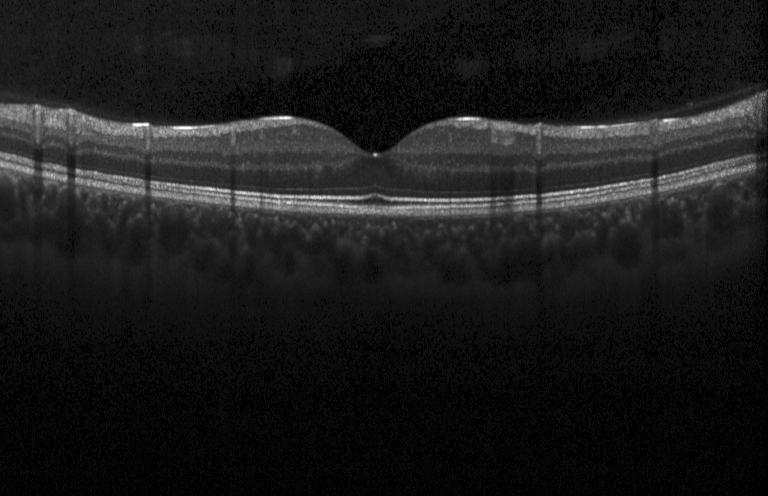

Impression: no evidence of choroidal neovascularization, diabetic macular edema, or drusen.